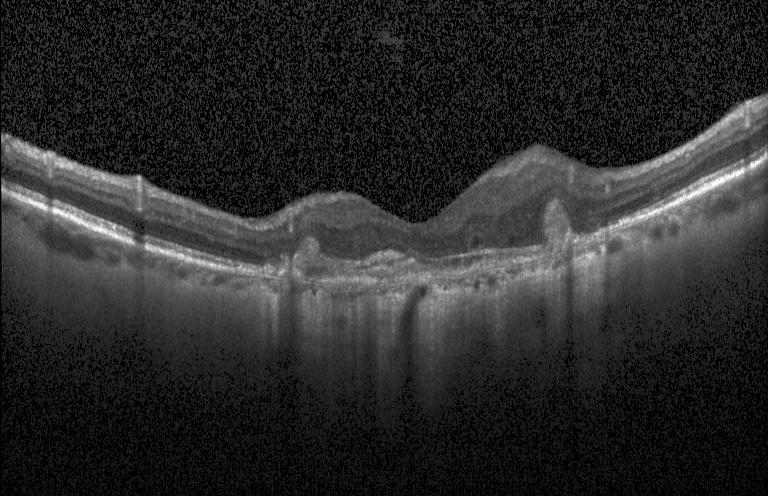
Macular OCT demonstrating a choroidal neovascular membrane.